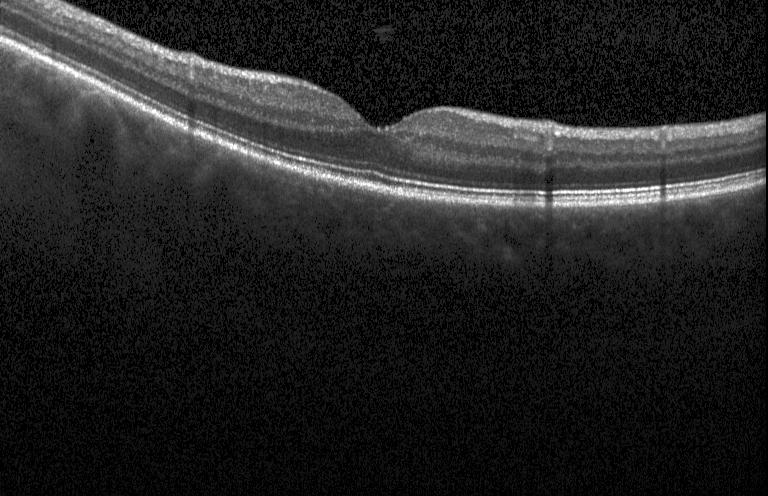 Macular OCT demonstrating no CNV, DME, or drusen.